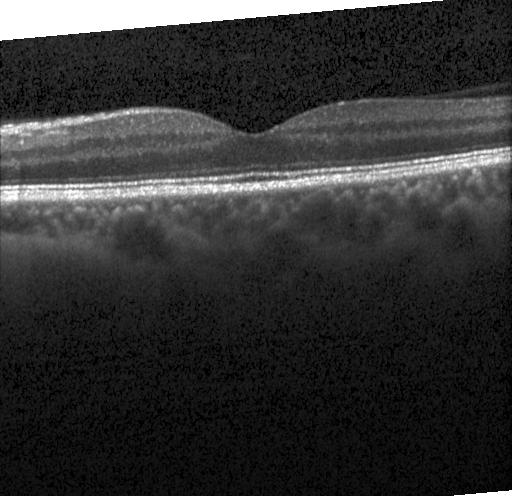 Impression: no choroidal neovascularization, diabetic macular edema, or drusen.